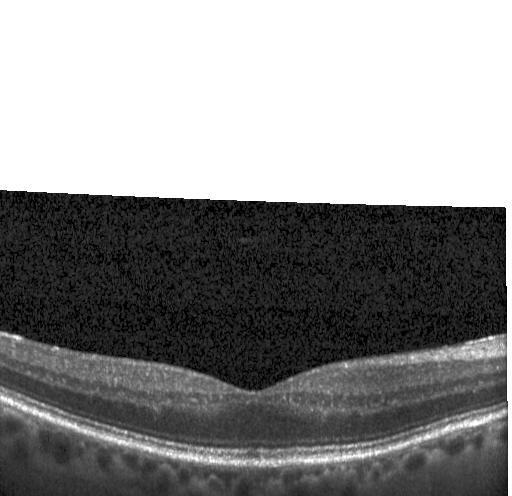

Finding: no choroidal neovascularization, diabetic macular edema, or drusen.